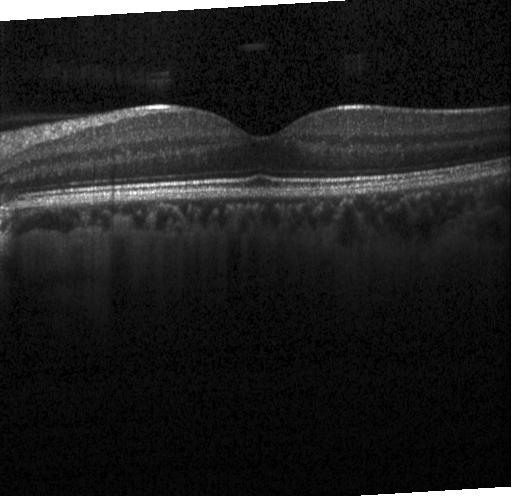
Optical coherence tomography scan — Assessment: no evidence of CNV, DME, or drusen.